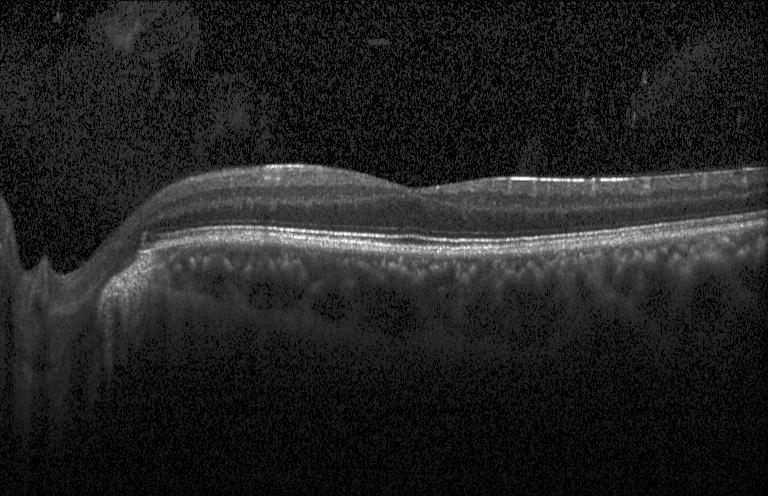 Spectral-domain OCT; optical coherence tomography scan
Macular OCT: no choroidal neovascularization, no diabetic macular edema, and no drusen.